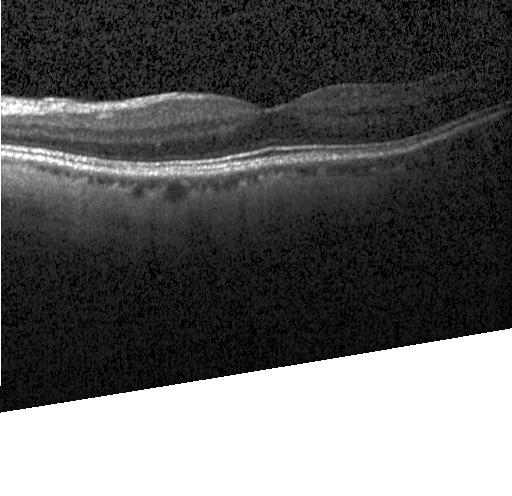

Heidelberg Spectralis, macular scan, OCT line scan.
Assessment: no choroidal neovascularization, no diabetic macular edema, and no drusen.